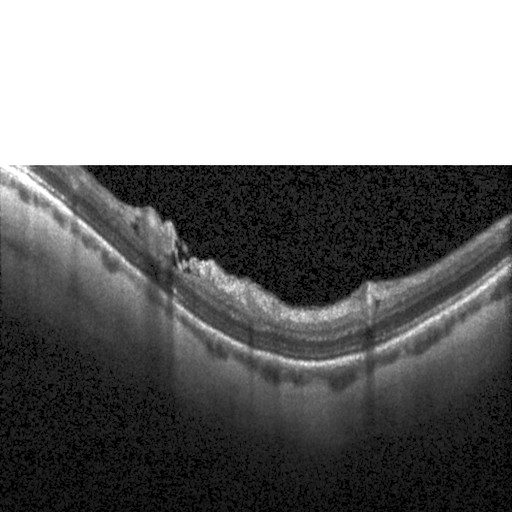
Spectral-domain OCT. Retinal OCT B-scan. Macular scan. Heidelberg Spectralis OCT system.
DME.